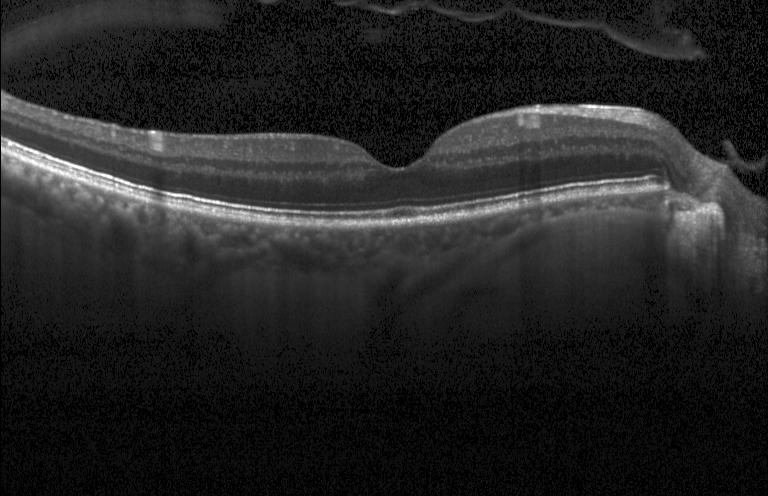 Horizontal scan through the fovea; spectral-domain OCT; acquired on a Heidelberg Spectralis; optical coherence tomography scan. Diagnosis: neither choroidal neovascularization, diabetic macular edema, nor drusen.